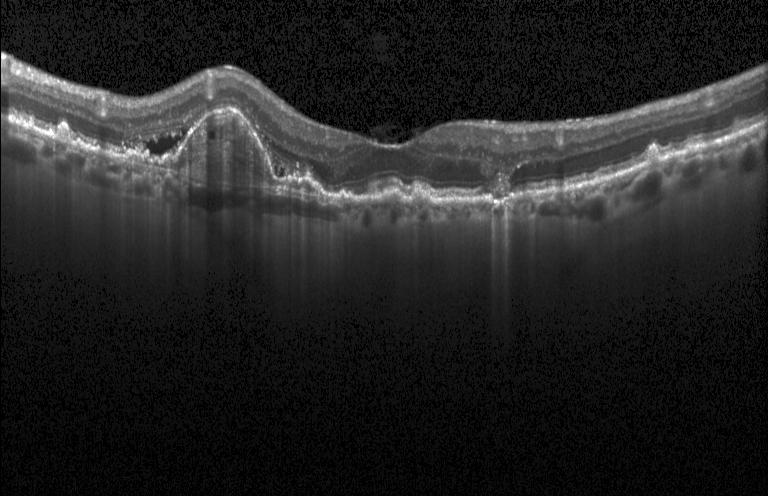
Retinal OCT cross-section. SD-OCT.
Diagnosis: a choroidal neovascular membrane.